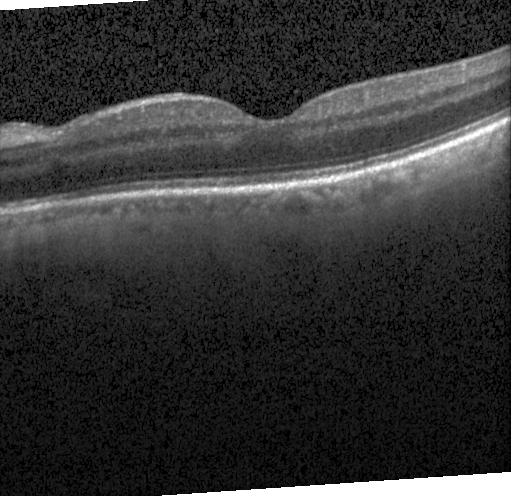

OCT finding: no choroidal neovascularization, diabetic macular edema, or drusen.